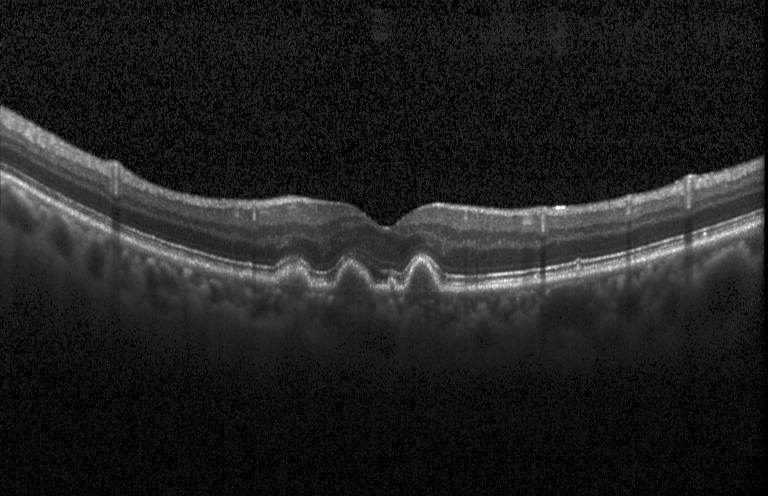
Retinal OCT cross-section — Impression: sub-RPE drusenoid deposits.